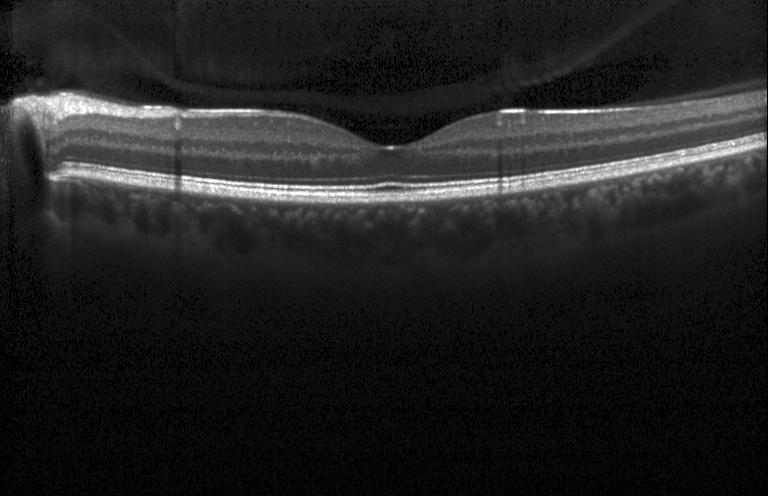 Impression: neither choroidal neovascularization, diabetic macular edema, nor drusen.